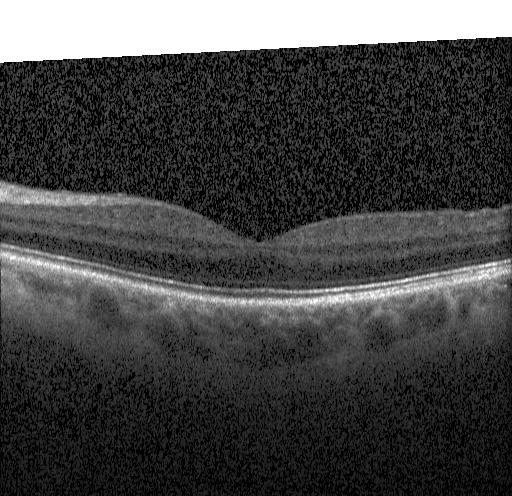

Macular OCT demonstrating no evidence of choroidal neovascularization, diabetic macular edema, or drusen.